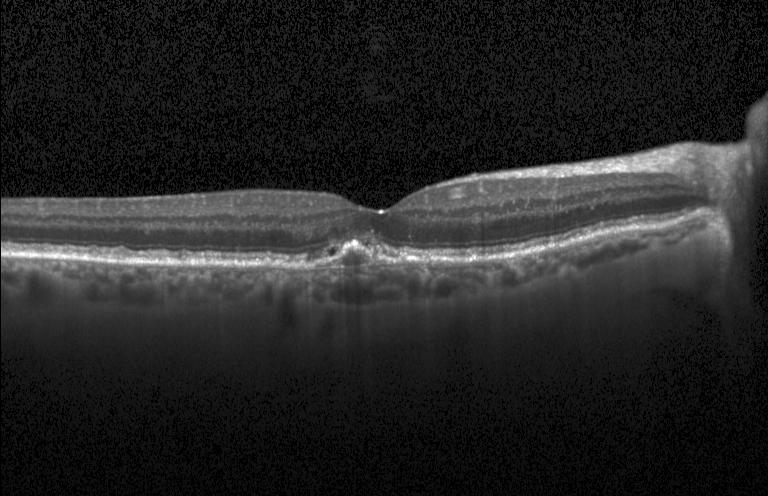 Optical coherence tomography scan. SD-OCT — CNV.